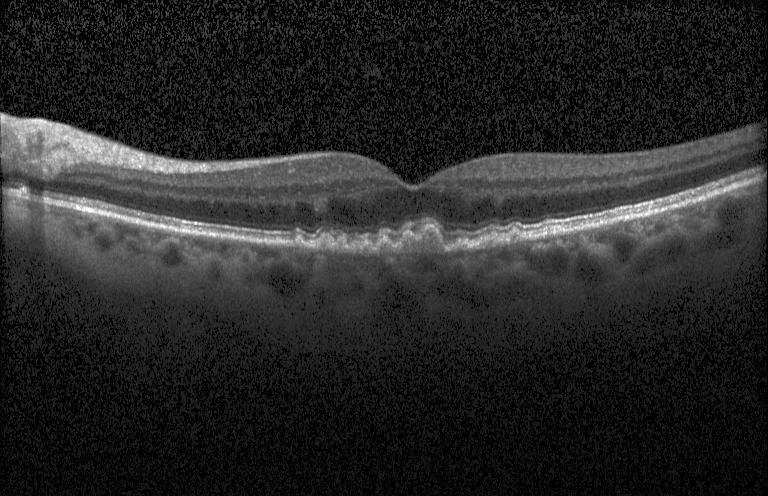

Finding: drusen.